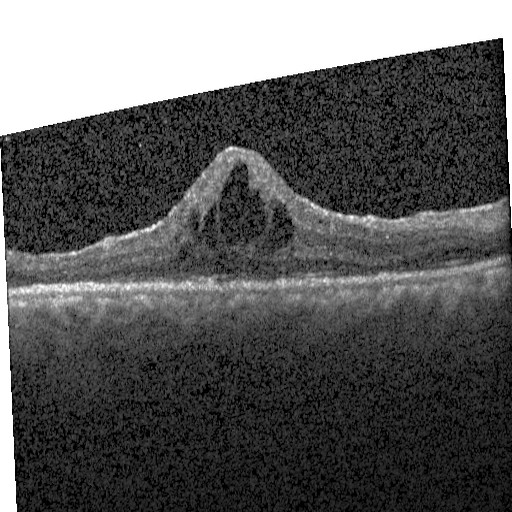 Optical coherence tomography scan.
Finding: diabetic macular edema.